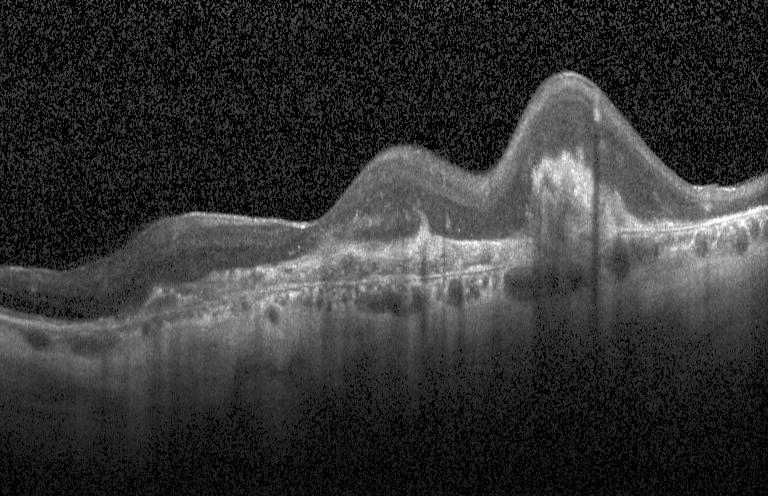

The scan shows CNV.